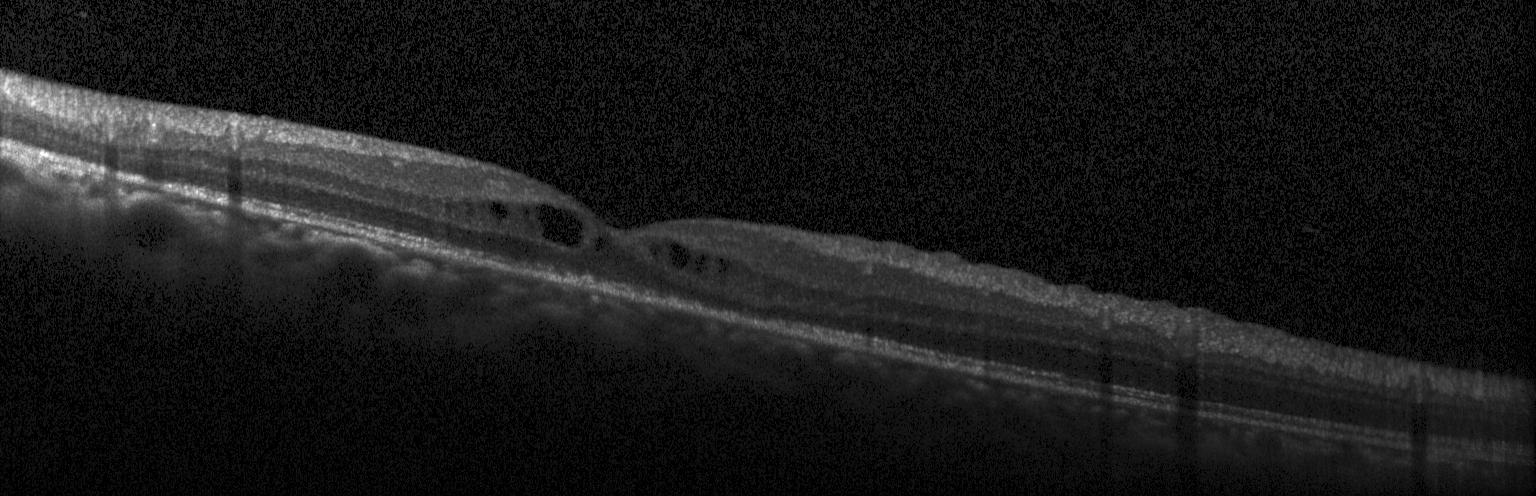

Spectral-domain optical coherence tomography, fovea-centered, OCT line scan. Assessment: diabetic macular edema.